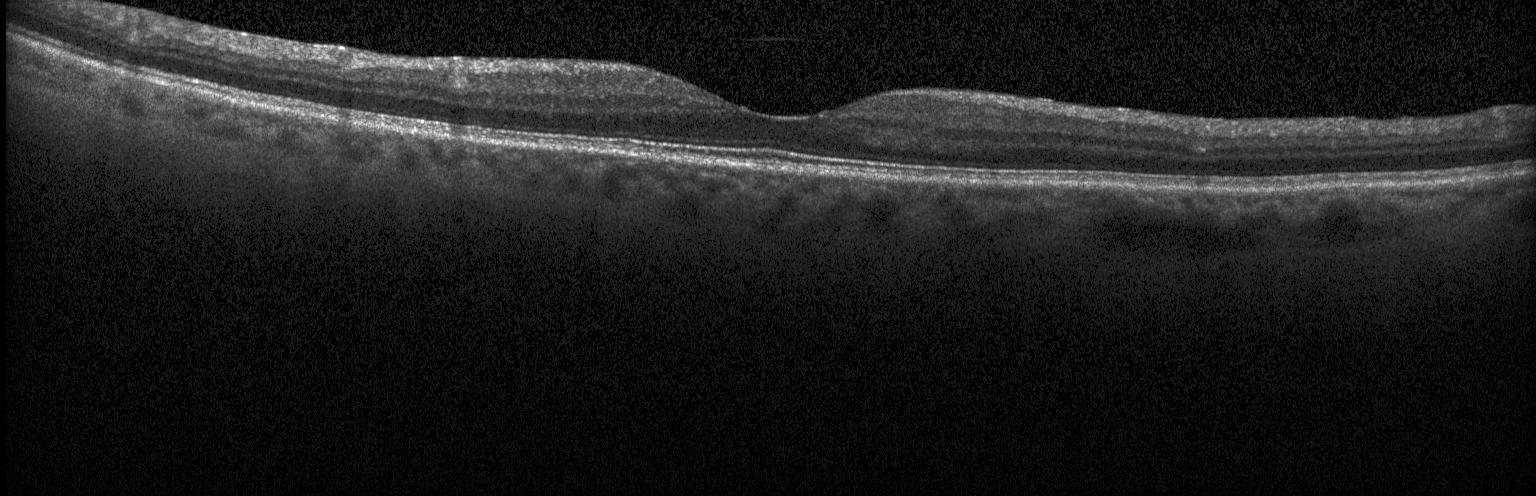

The scan shows no CNV, no DME, and no drusen.